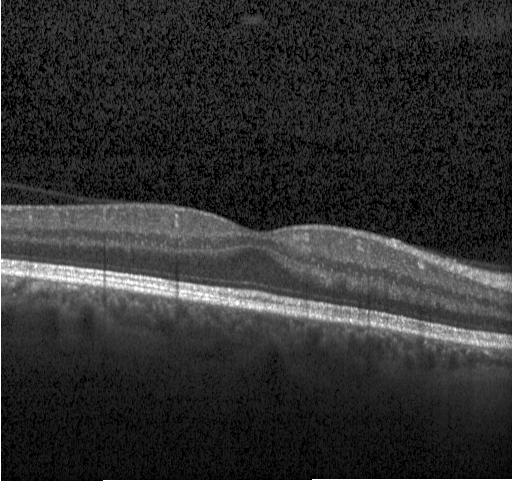 Fovea-centered; acquired on a Heidelberg Spectralis; OCT line scan.
The scan shows no choroidal neovascularization, diabetic macular edema, or drusen.